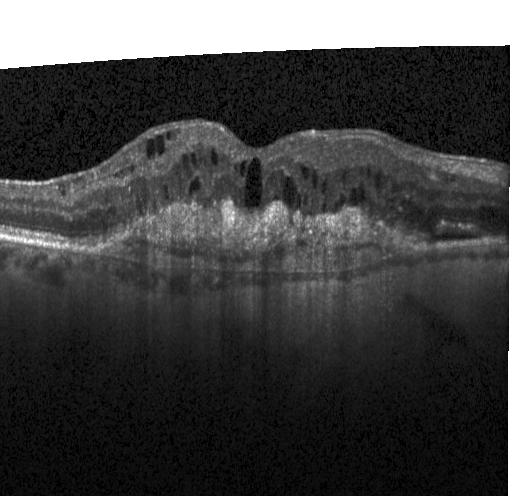 SD-OCT, acquired on a Heidelberg Spectralis, optical coherence tomography B-scan — Diagnosis: a choroidal neovascular membrane.